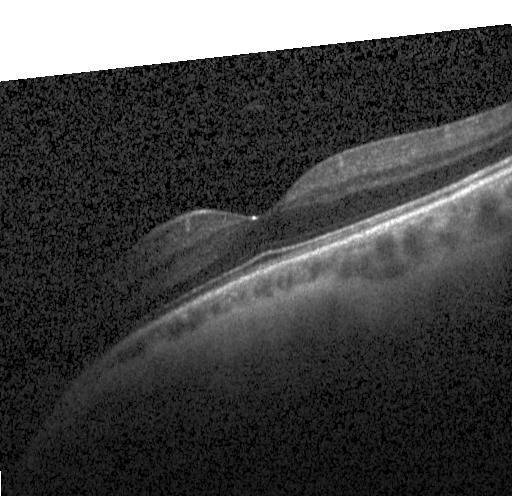

Spectral-domain optical coherence tomography. OCT B-scan
Finding: no evidence of CNV, DME, or drusen.